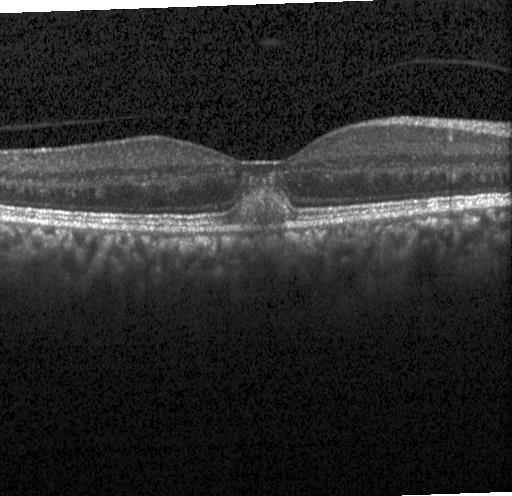

Diagnosis: a choroidal neovascular membrane.